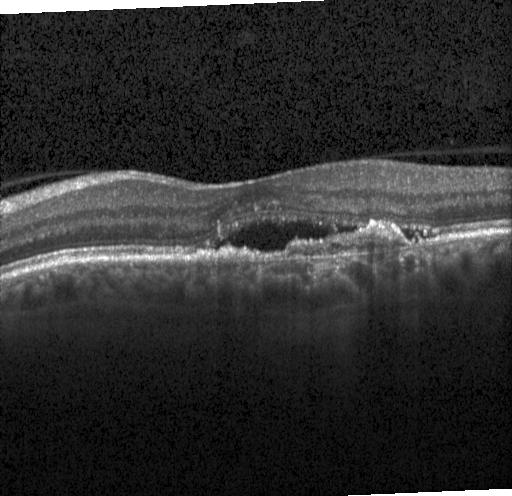

OCT line scan, spectral-domain optical coherence tomography, Heidelberg Spectralis.
The scan shows a choroidal neovascular membrane.